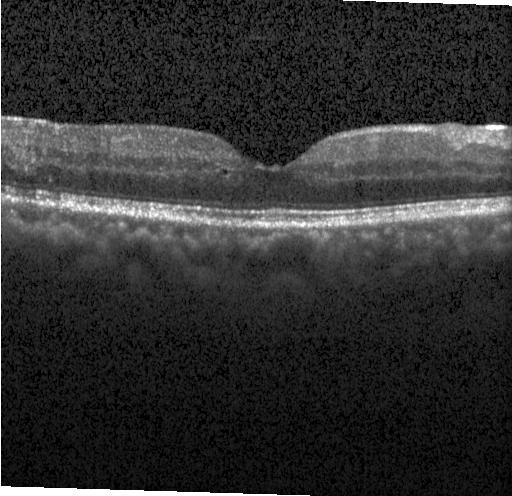

Spectral-domain optical coherence tomography. Centered on the fovea. Instrument: Heidelberg Spectralis. Retinal OCT cross-section. Impression: diabetic macular edema.